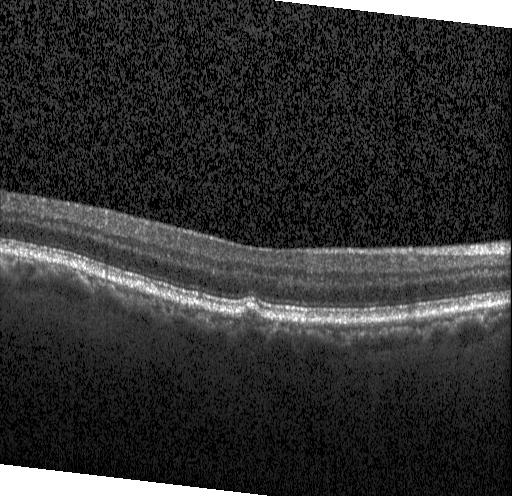 OCT line scan. Acquired on a Heidelberg Spectralis. Through the macula
Impression: sub-RPE drusenoid deposits.